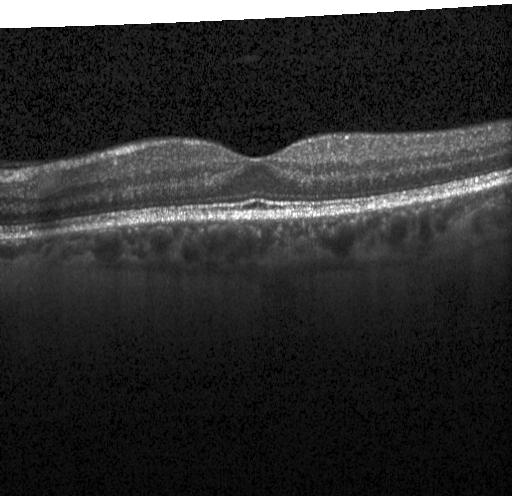

Macular OCT: neither CNV, DME, nor drusen.